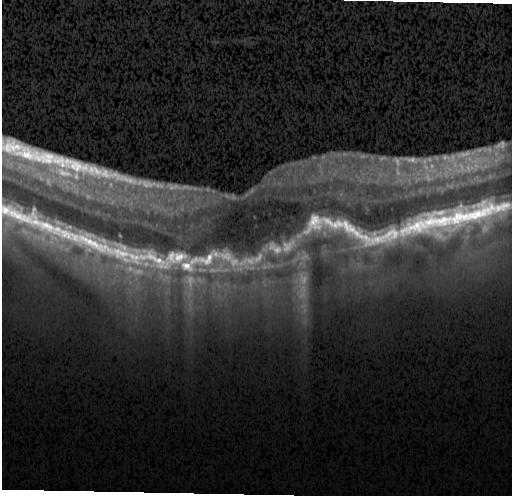

Finding: a choroidal neovascular membrane.